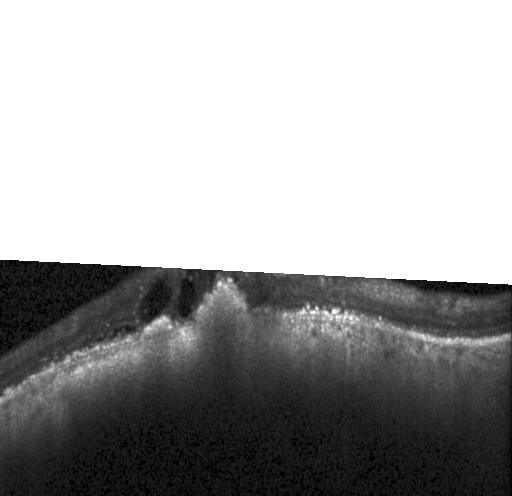 Impression: choroidal neovascularization (CNV).